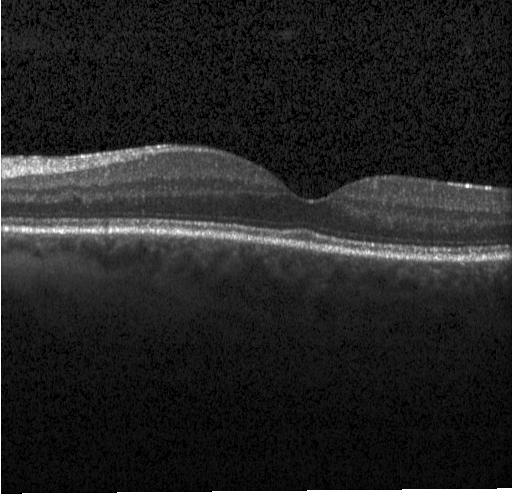

Through the macula, acquired on a Heidelberg Spectralis, SD-OCT, optical coherence tomography B-scan.
Finding: neither choroidal neovascularization, diabetic macular edema, nor drusen.